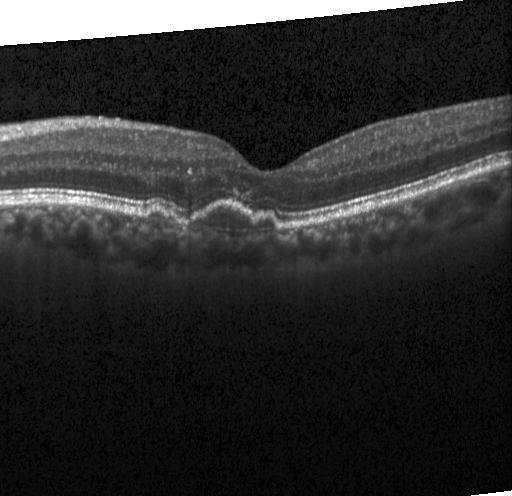
Spectral-domain OCT. Retinal OCT B-scan. Instrument: Heidelberg Spectralis. Macular scan
Impression: choroidal neovascularization.